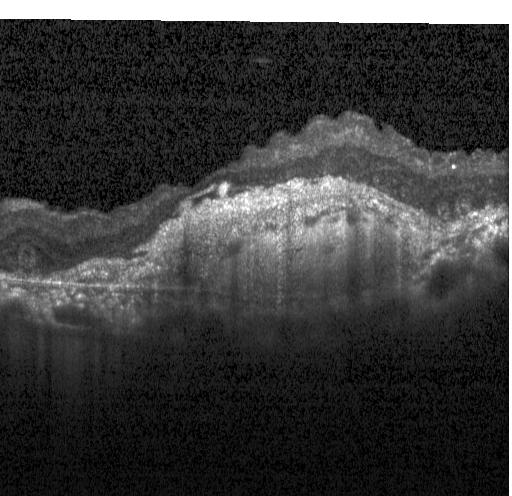
Optical coherence tomography scan — This B-scan demonstrates choroidal neovascularization.